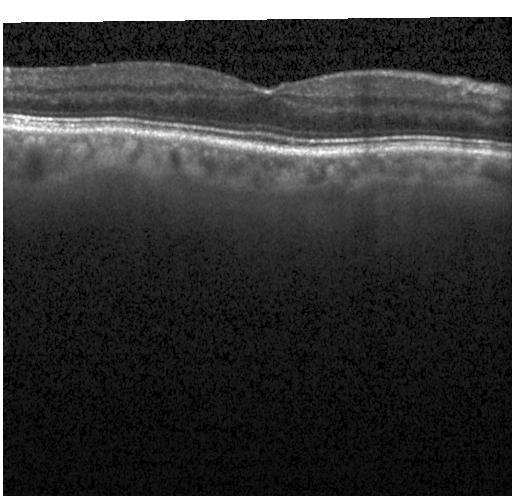
Retinal OCT cross-section showing no CNV, no DME, and no drusen.